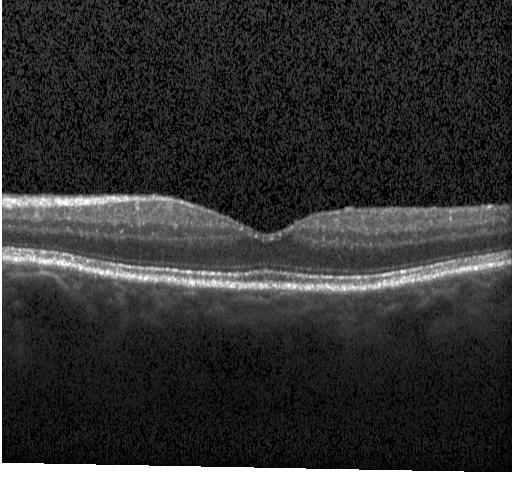
Spectral-domain OCT B-scan: neither CNV, DME, nor drusen.